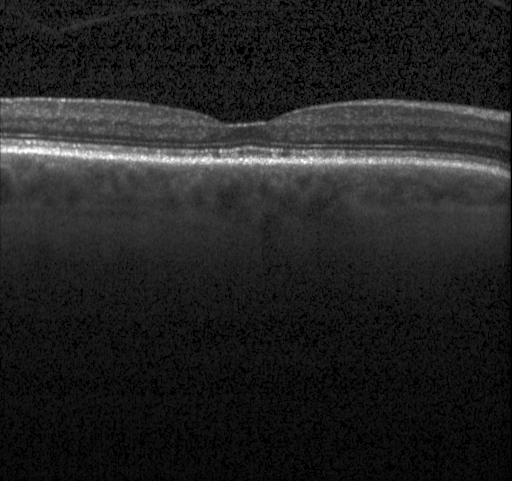
Centered on the fovea, OCT line scan, spectral-domain OCT. The scan shows neither CNV, DME, nor drusen.